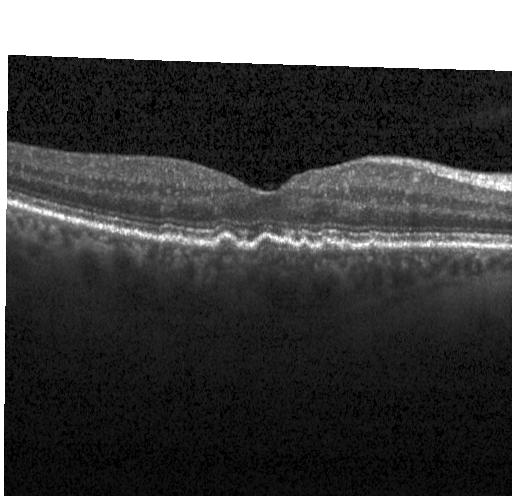 OCT finding: multiple drusen.